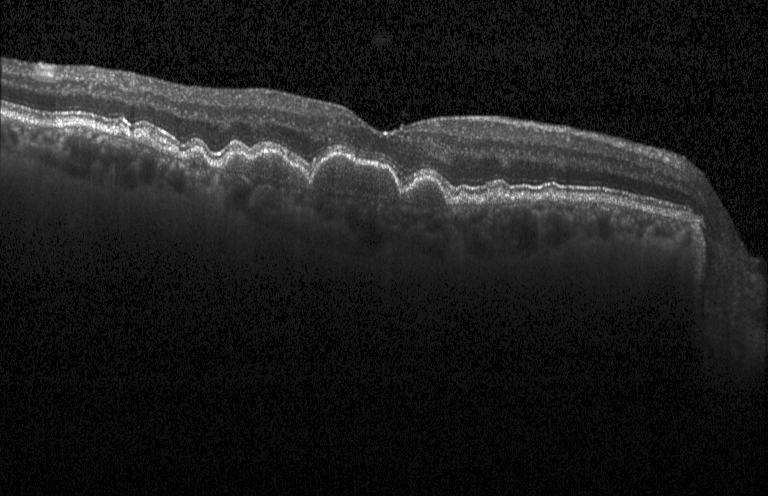

Impression: sub-RPE drusenoid deposits.